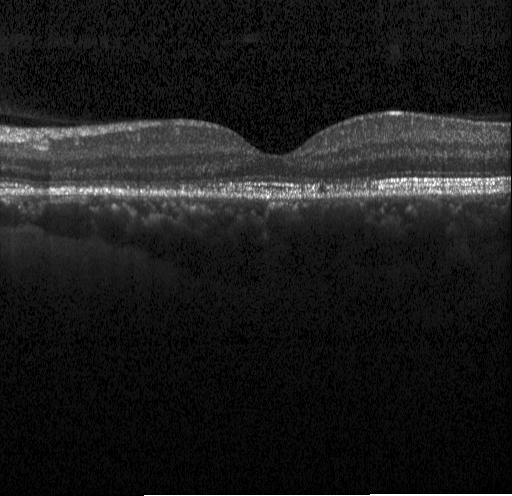 Retinal OCT cross-section
OCT finding: no evidence of choroidal neovascularization, diabetic macular edema, or drusen.